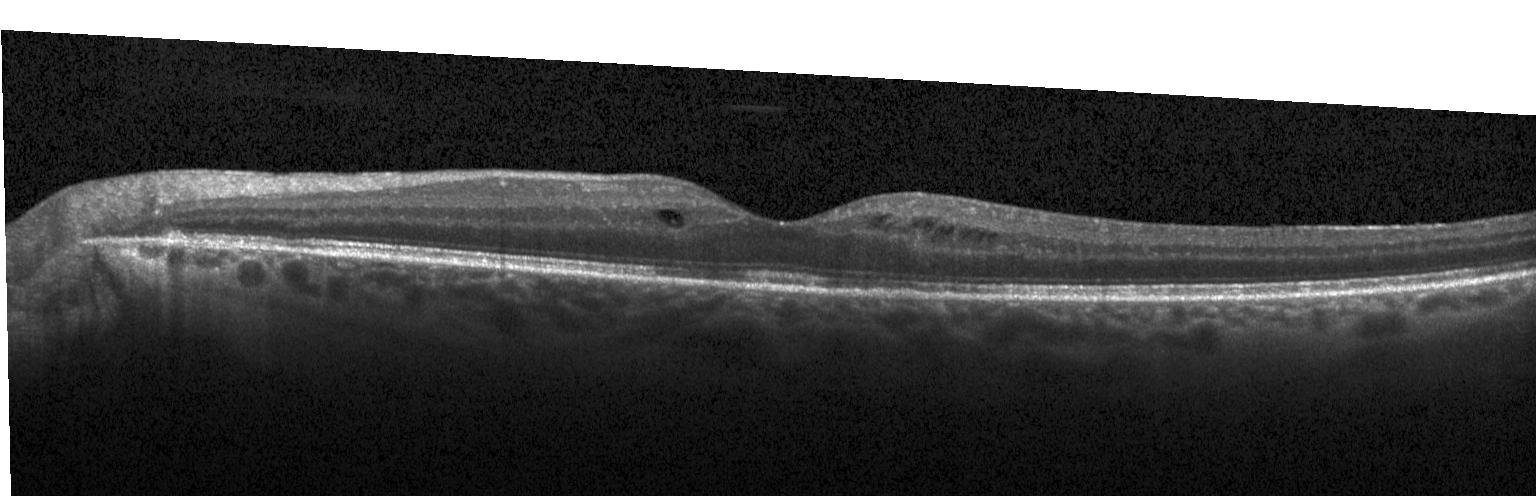

Spectral-domain optical coherence tomography · optical coherence tomography B-scan — Finding: diabetic macular edema.